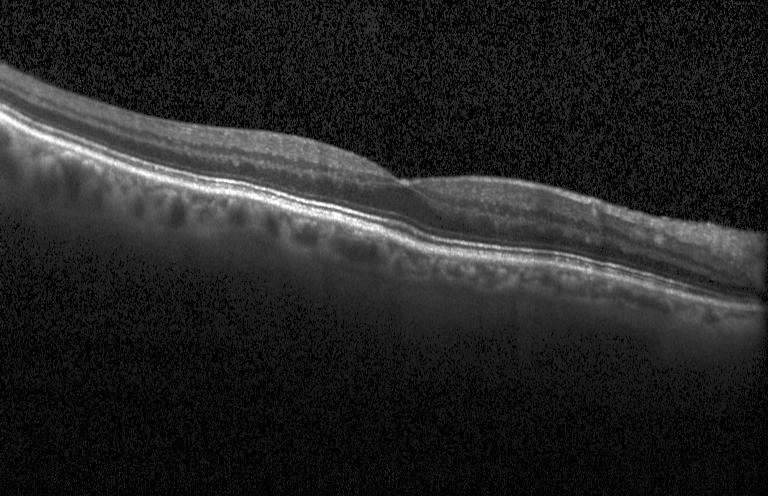 Macular OCT demonstrating no evidence of choroidal neovascularization, diabetic macular edema, or drusen.